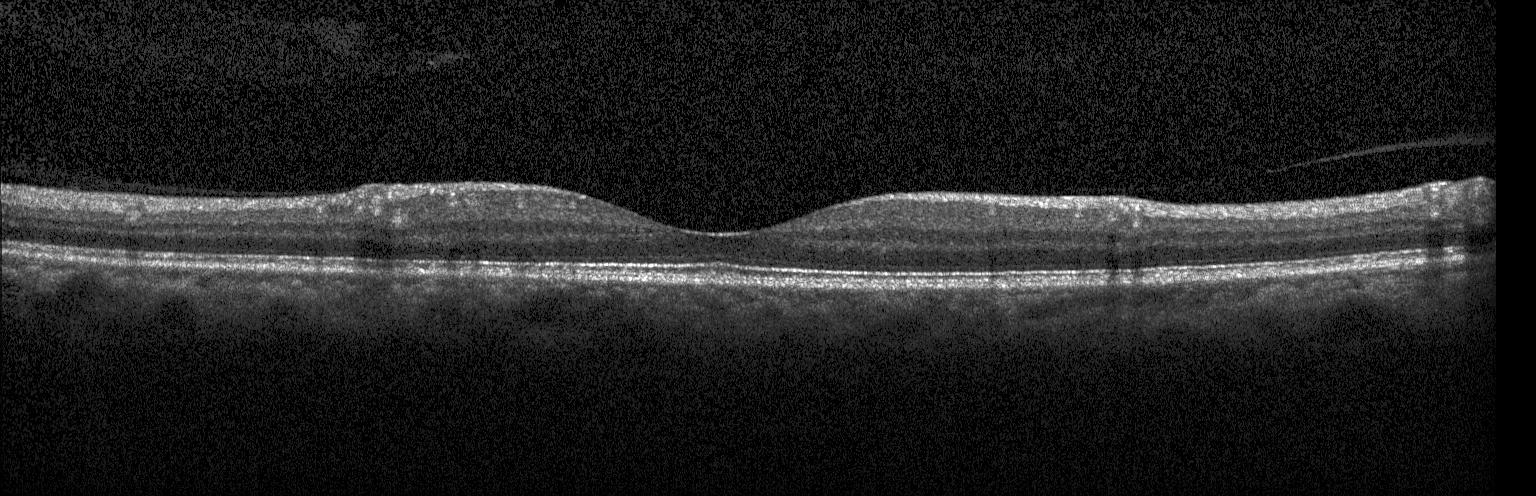 SD-OCT, optical coherence tomography B-scan, Heidelberg Spectralis. Finding: no choroidal neovascularization, no diabetic macular edema, and no drusen.